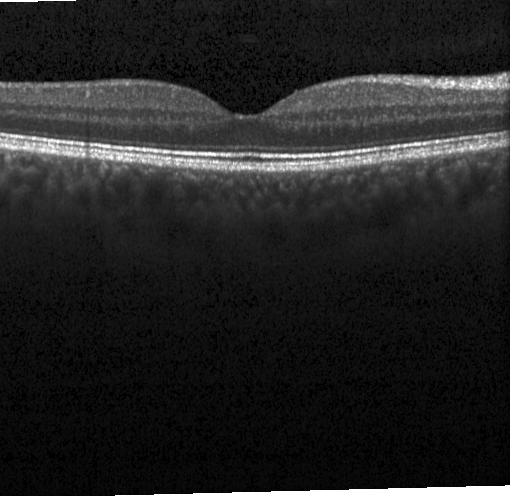 Impression: no evidence of CNV, DME, or drusen.